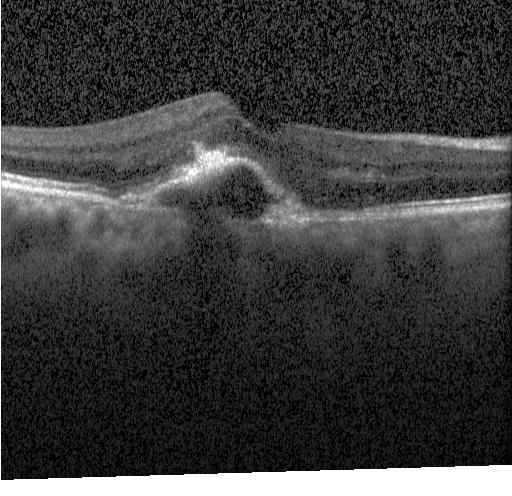

Impression: choroidal neovascularization (CNV).